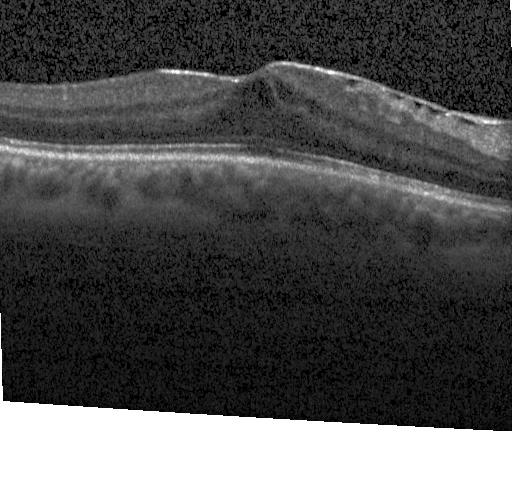 Optical coherence tomography scan. Horizontal scan through the fovea
Impression: DME.